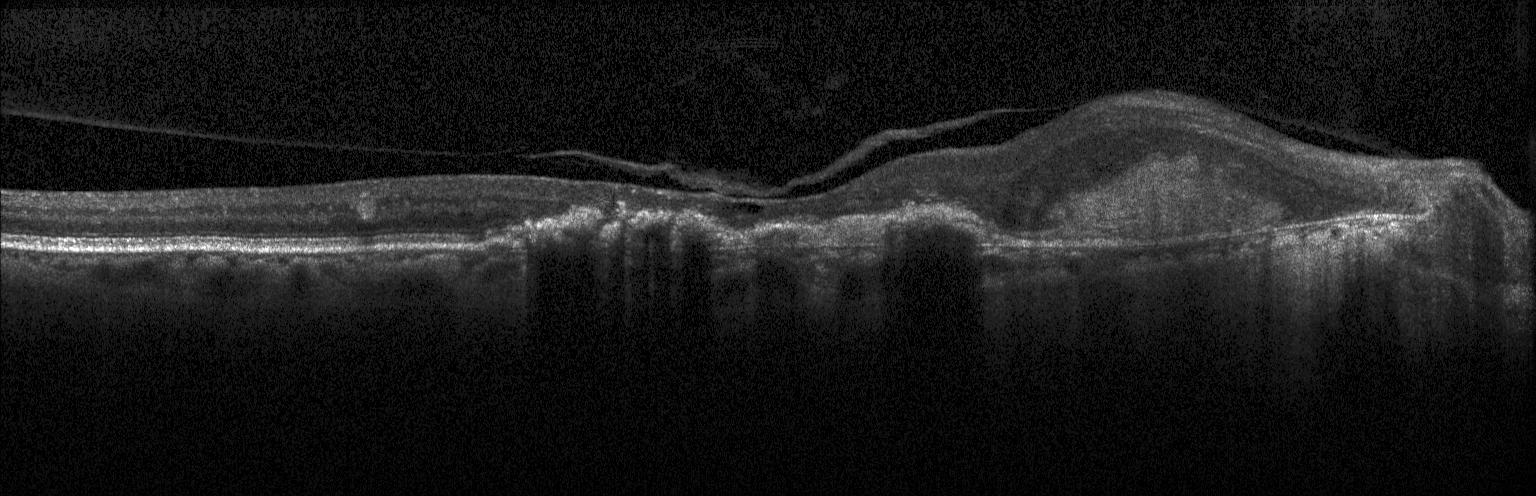
Acquired on a Heidelberg Spectralis. Horizontal scan through the fovea. Spectral-domain optical coherence tomography. Retinal OCT B-scan
Finding: a choroidal neovascular membrane.